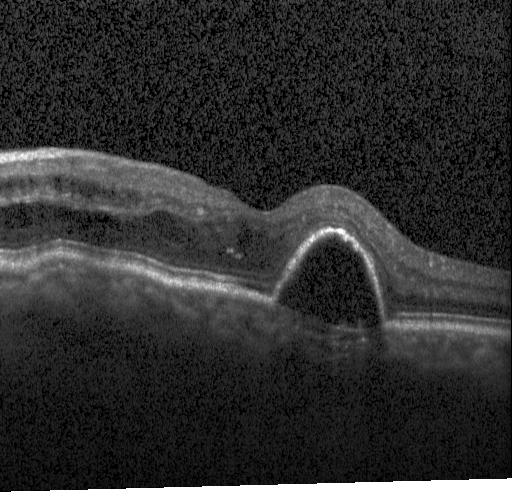
Optical coherence tomography B-scan.
Assessment: a choroidal neovascular membrane.